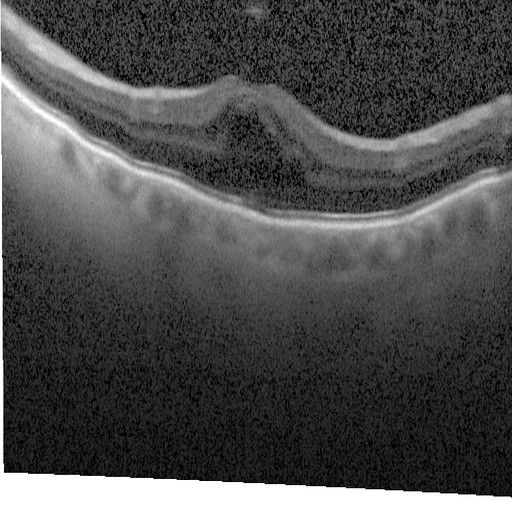
Optical coherence tomography scan.
Diagnosis: diabetic macular edema (DME).